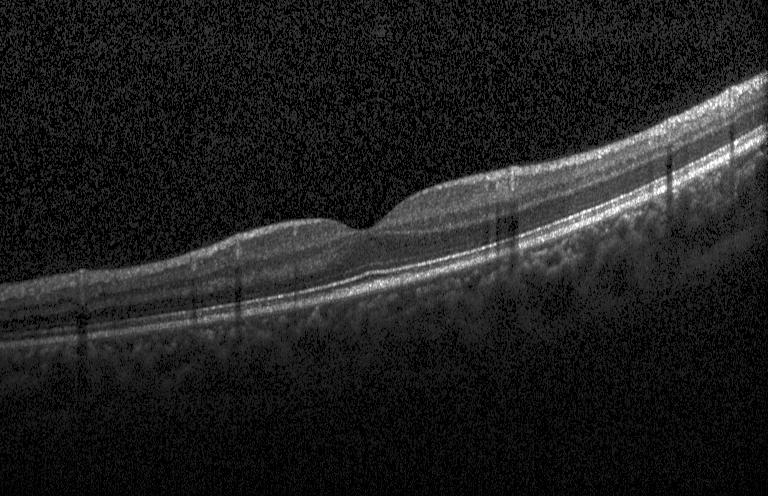 Retinal OCT cross-section · acquired on a Heidelberg Spectralis · macular scan.
Diagnosis: no evidence of CNV, DME, or drusen.